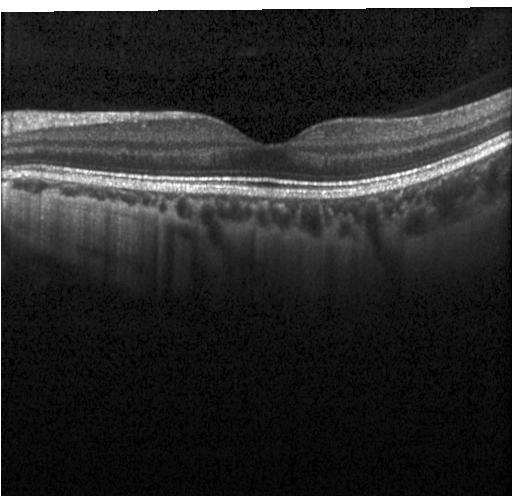

Through the macula. SD-OCT. Optical coherence tomography B-scan. Instrument: Heidelberg Spectralis
Finding: no CNV, no DME, and no drusen.